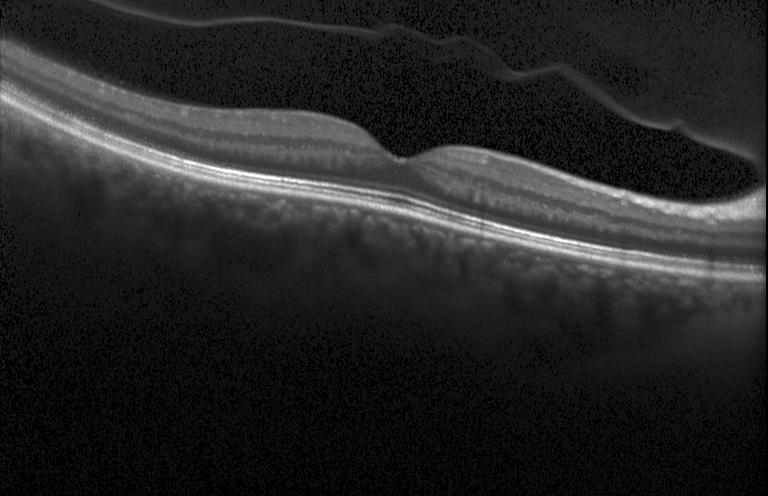 Retinal OCT cross-section showing no choroidal neovascularization, diabetic macular edema, or drusen.